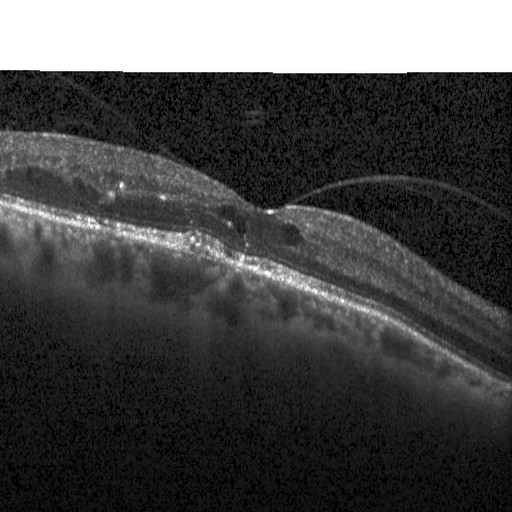

OCT scan showing DME.